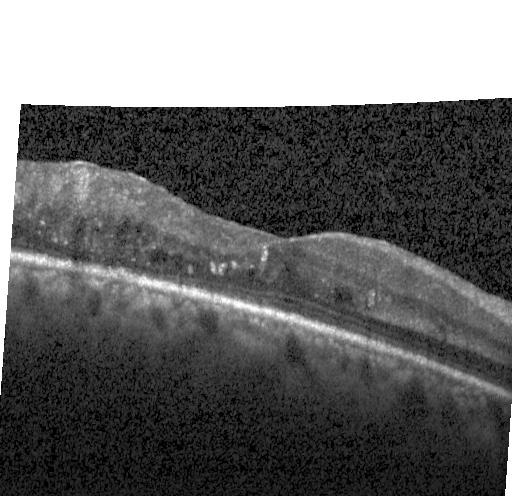 Retinal OCT cross-section showing DME.